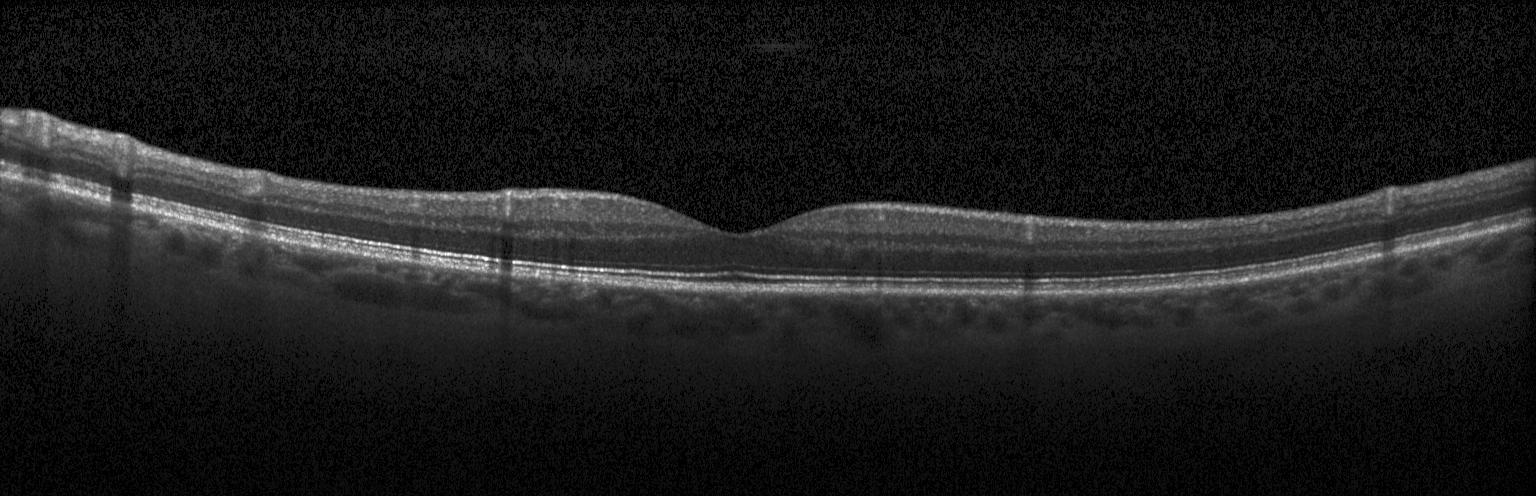 This B-scan demonstrates neither CNV, DME, nor drusen.